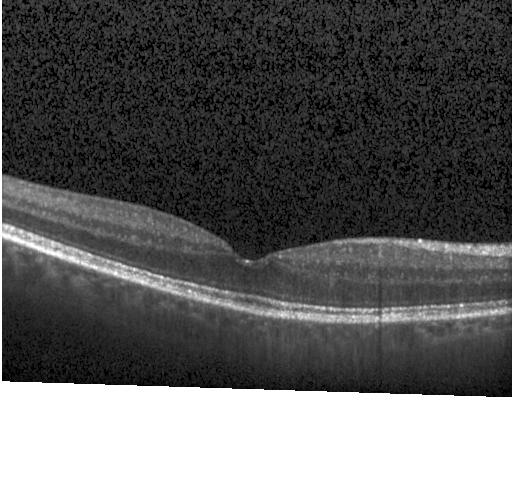

OCT finding: no evidence of CNV, DME, or drusen.